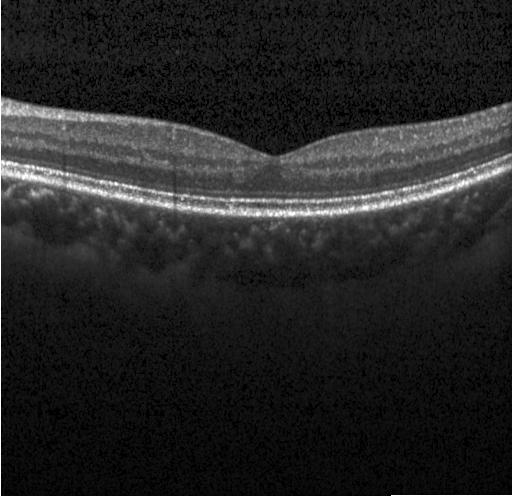
Instrument: Heidelberg Spectralis · OCT line scan · SD-OCT · macular scan
The scan shows no CNV, no DME, and no drusen.